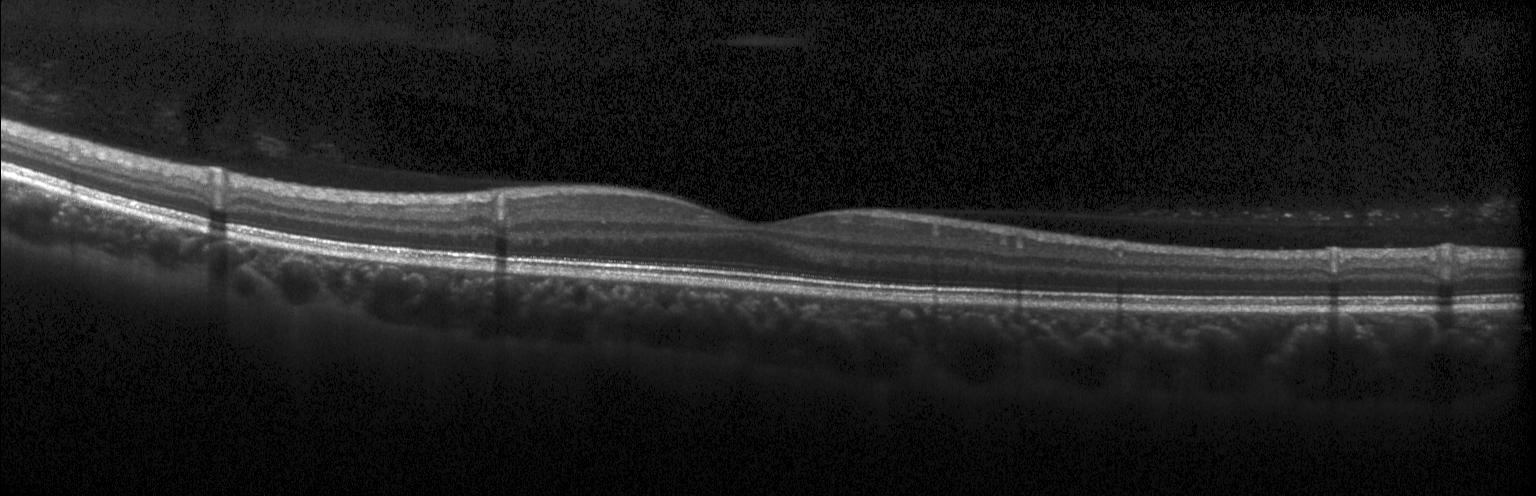

Instrument: Heidelberg Spectralis, SD-OCT, OCT B-scan, macular scan. Assessment: neither choroidal neovascularization, diabetic macular edema, nor drusen.